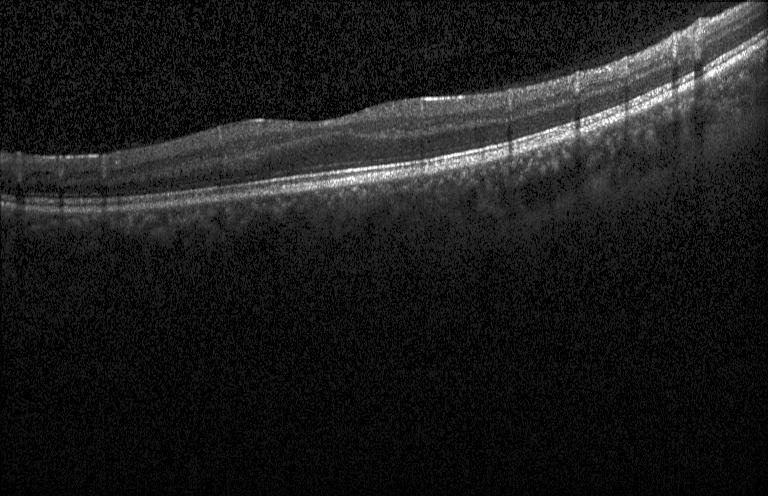
Impression: no evidence of CNV, DME, or drusen.